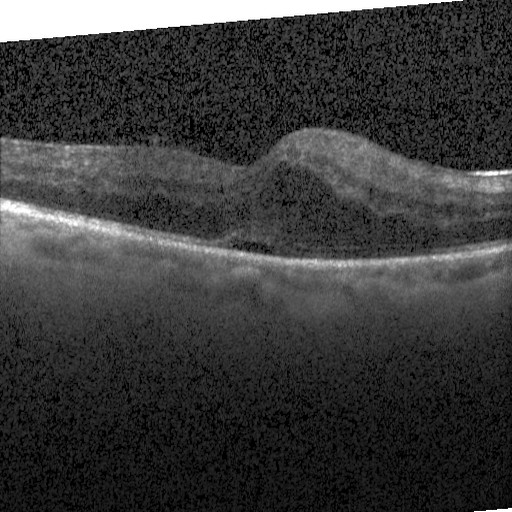
Macular scan. Retinal OCT B-scan. Acquired on a Heidelberg Spectralis. Spectral-domain optical coherence tomography. Finding: diabetic macular edema (DME).